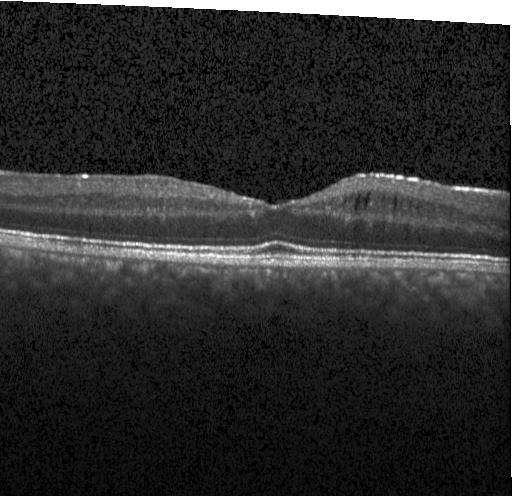 Optical coherence tomography B-scan. Heidelberg Spectralis
Dx: diabetic macular edema.